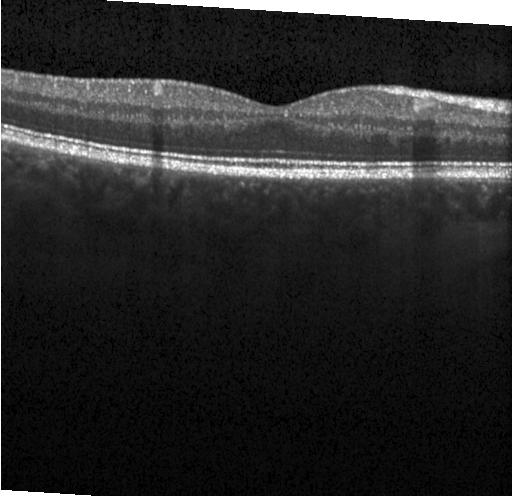
Finding: no choroidal neovascularization, diabetic macular edema, or drusen.